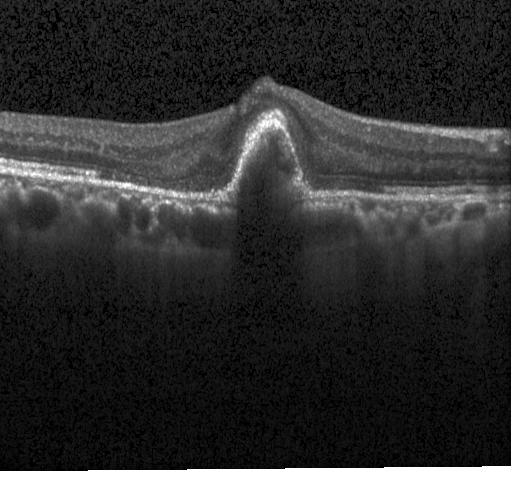
Fovea-centered; spectral-domain optical coherence tomography; optical coherence tomography B-scan; Heidelberg Spectralis. Impression: CNV.